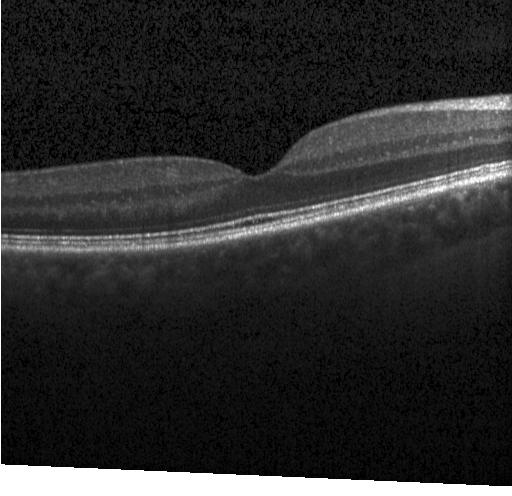 Retinal OCT B-scan, Heidelberg Spectralis
Finding: no choroidal neovascularization, diabetic macular edema, or drusen.